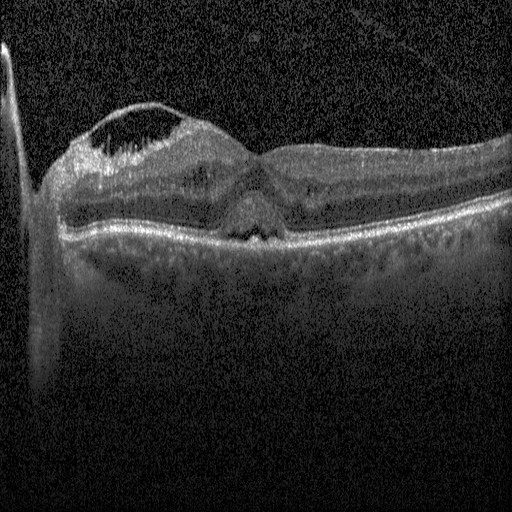 Optical coherence tomography B-scan; spectral-domain optical coherence tomography; macular scan. This B-scan demonstrates DME.